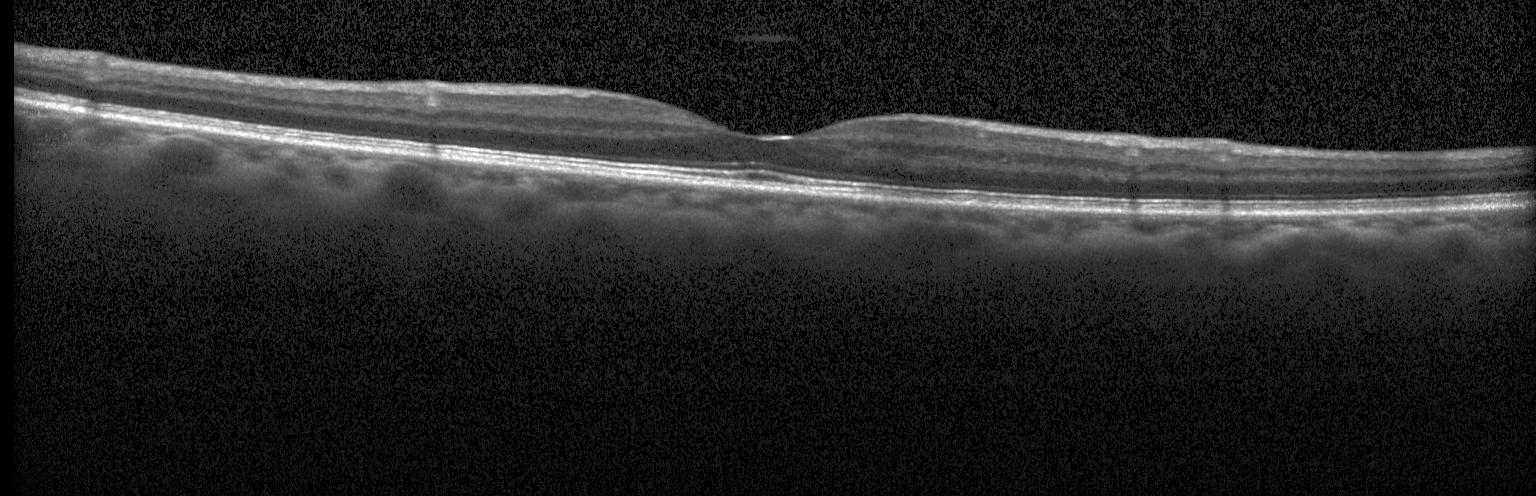
Optical coherence tomography scan. No evidence of choroidal neovascularization, diabetic macular edema, or drusen.